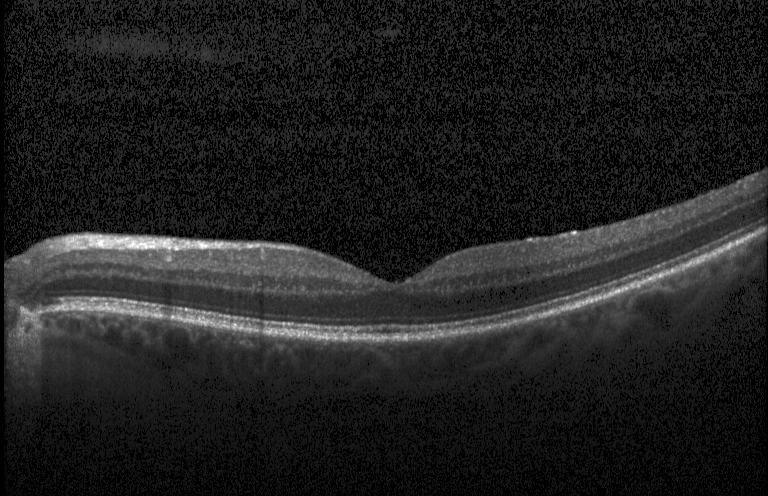
Optical coherence tomography B-scan. Heidelberg Spectralis OCT system
The scan shows no choroidal neovascularization, no diabetic macular edema, and no drusen.